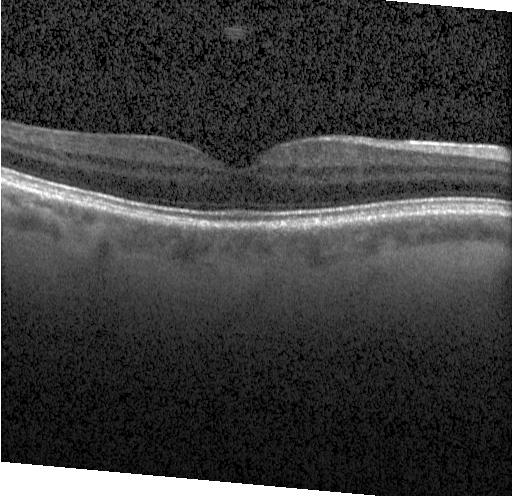
OCT B-scan. Finding: no choroidal neovascularization, diabetic macular edema, or drusen.